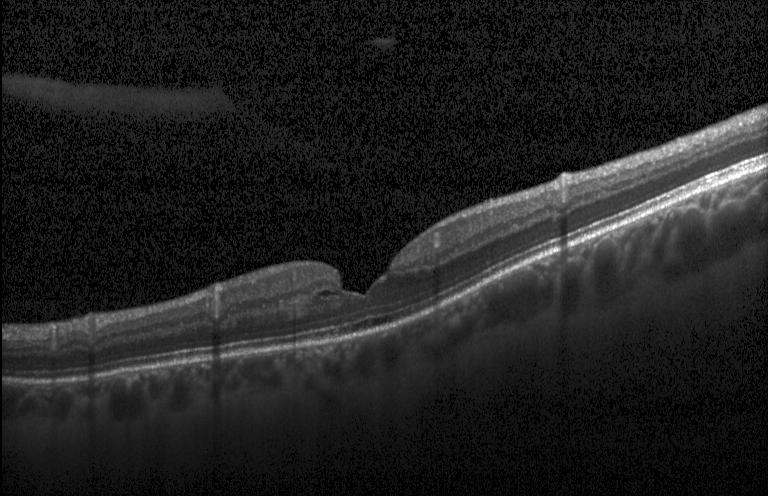 Heidelberg Spectralis OCT system · SD-OCT · OCT B-scan · centered on the fovea
Diagnosis: DME.